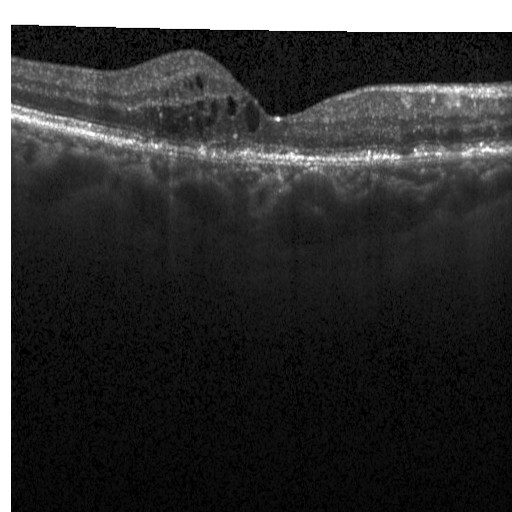
Instrument: Heidelberg Spectralis · SD-OCT · optical coherence tomography B-scan · centered on the fovea — Macular OCT: DME.